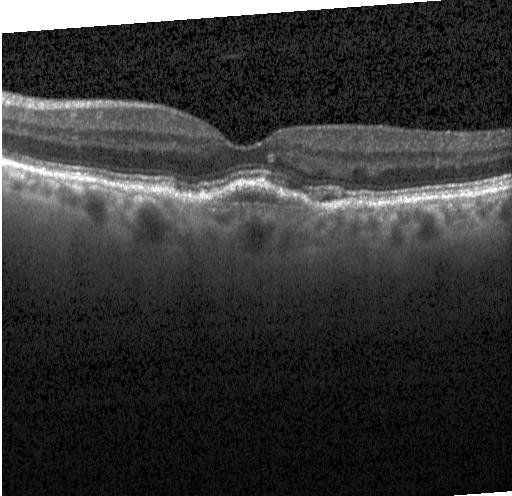 Retinal OCT cross-section, spectral-domain OCT, centered on the fovea.
Impression: a choroidal neovascular membrane.